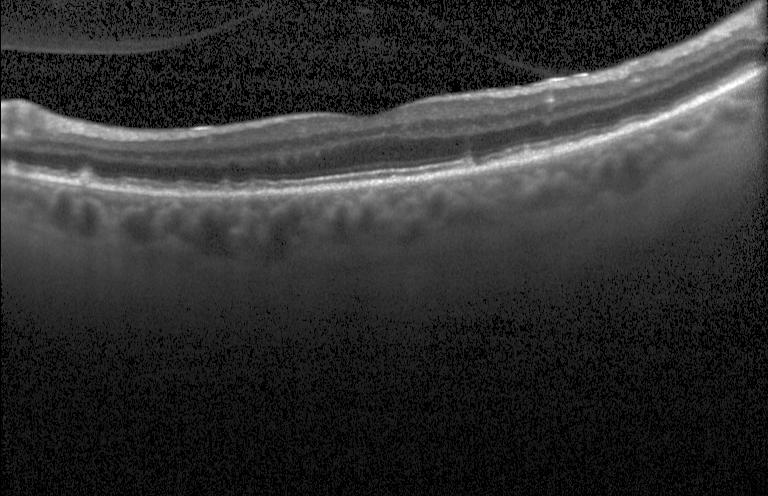 Optical coherence tomography scan — OCT finding: no choroidal neovascularization, diabetic macular edema, or drusen.